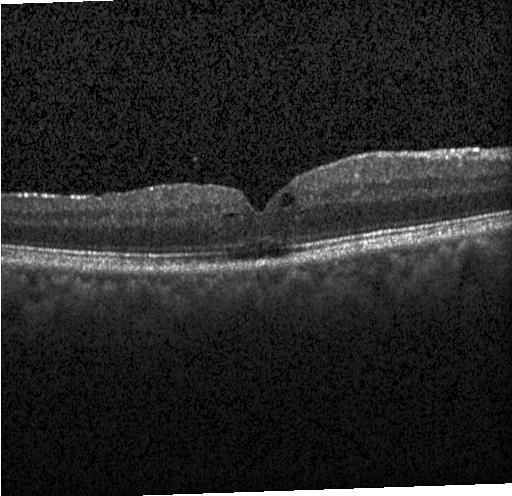

Spectral-domain OCT. Optical coherence tomography scan.
Impression: DME.